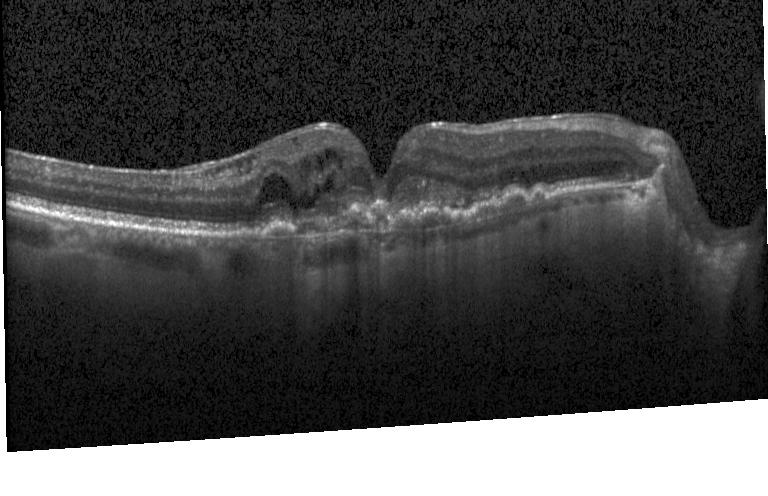
Heidelberg Spectralis OCT system · OCT line scan. Impression: a choroidal neovascular membrane.